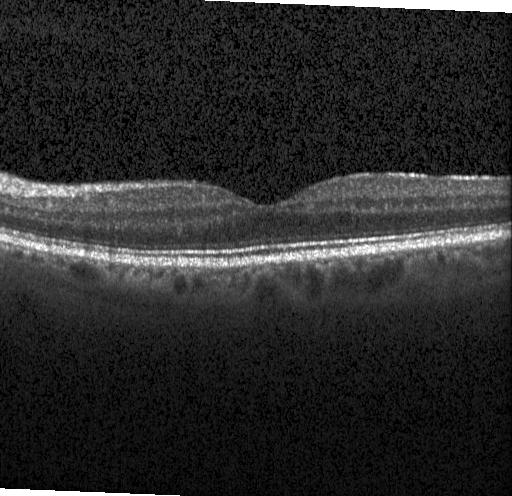 OCT B-scan
Diagnosis: no evidence of CNV, DME, or drusen.